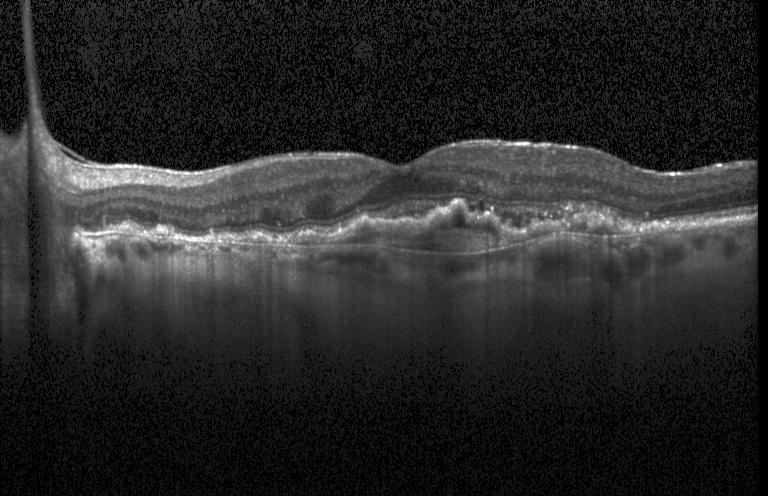
Instrument: Heidelberg Spectralis · retinal OCT cross-section · spectral-domain optical coherence tomography. Diagnosis: a choroidal neovascular membrane.